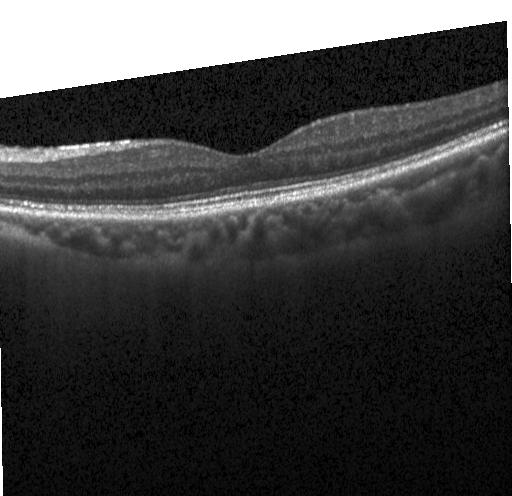
Fovea-centered. Optical coherence tomography scan. Heidelberg Spectralis. No choroidal neovascularization, diabetic macular edema, or drusen.